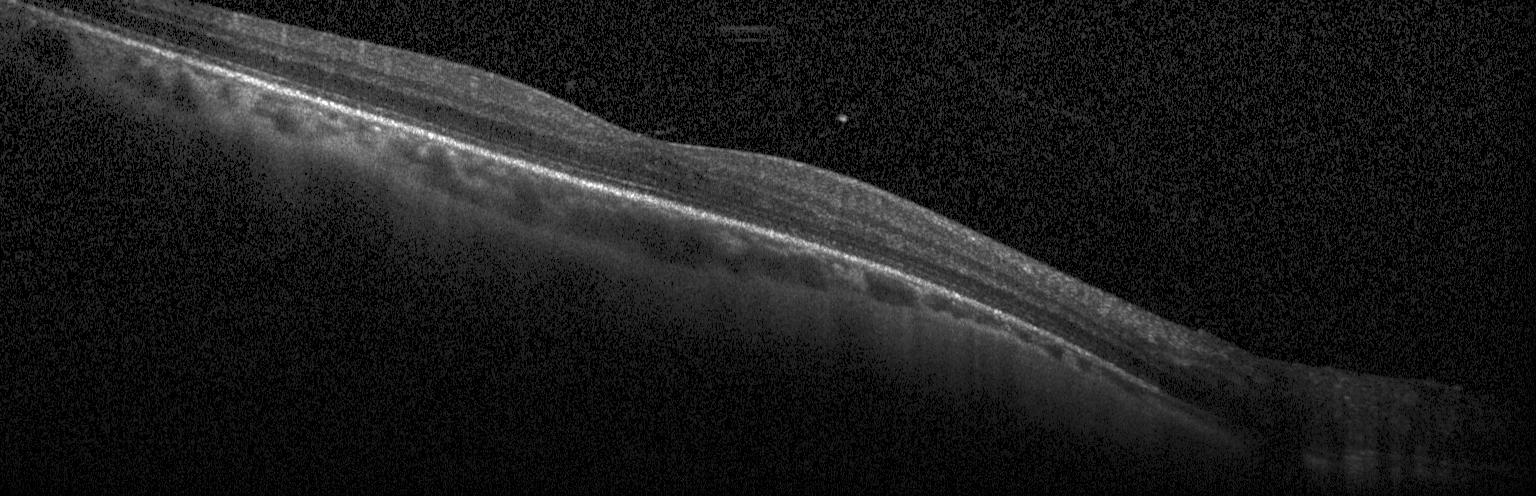

Retinal OCT cross-section showing neither CNV, DME, nor drusen.